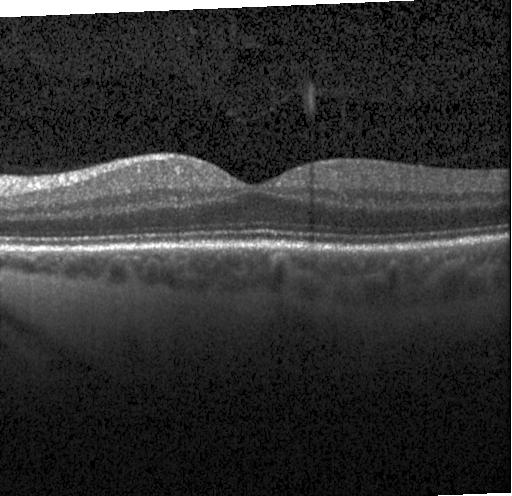
OCT line scan. Heidelberg Spectralis OCT system. Fovea-centered.
Macular OCT: no CNV, no DME, and no drusen.